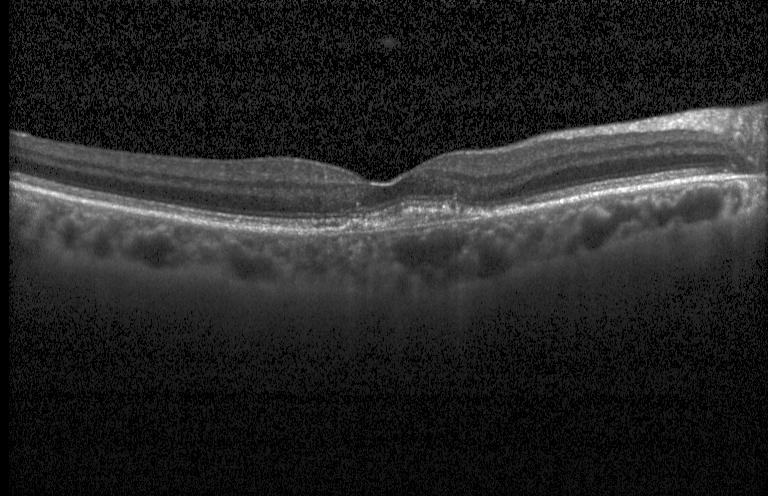
Spectral-domain OCT B-scan: choroidal neovascularization.